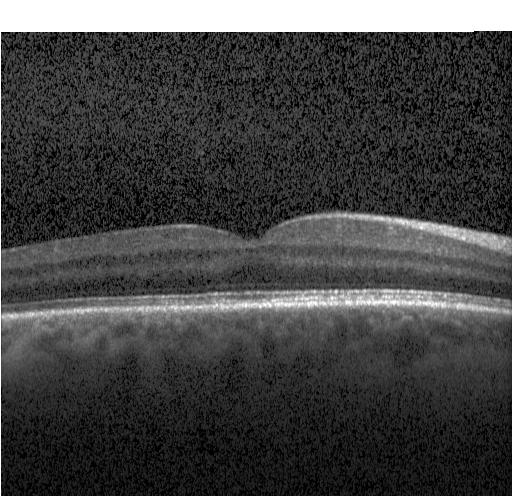

Heidelberg Spectralis. OCT B-scan — The scan shows no CNV, DME, or drusen.